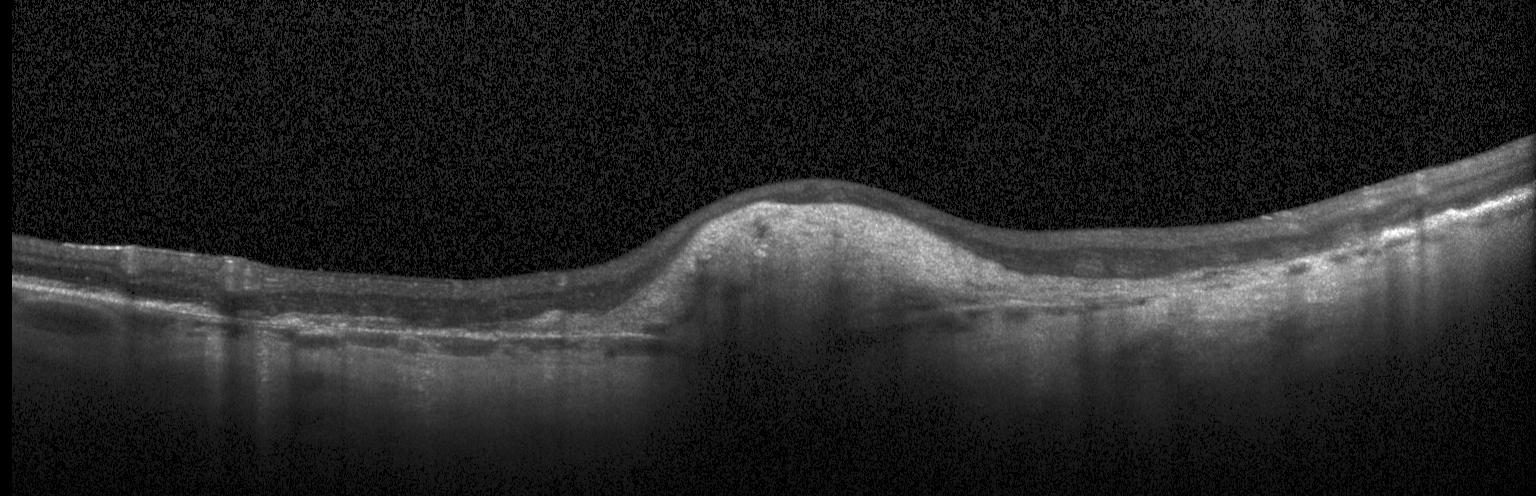

Centered on the fovea. Spectral-domain OCT. Retinal OCT cross-section — This B-scan demonstrates choroidal neovascularization (CNV).